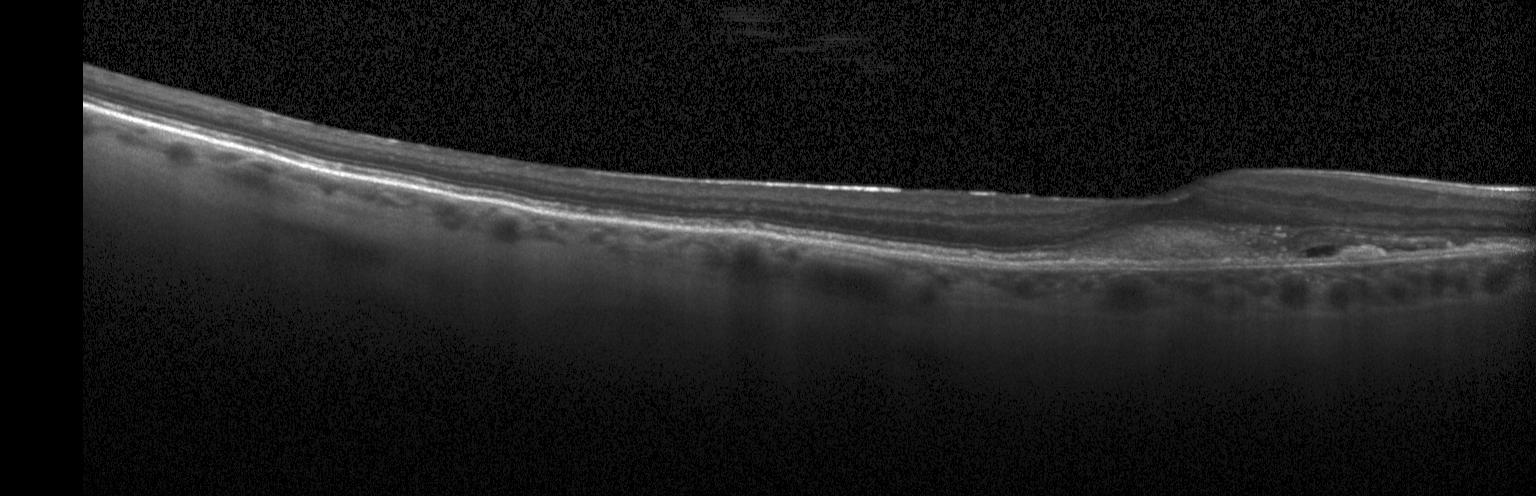 Retinal OCT cross-section. Instrument: Heidelberg Spectralis. Fovea-centered. Spectral-domain optical coherence tomography.
Impression: a choroidal neovascular membrane.